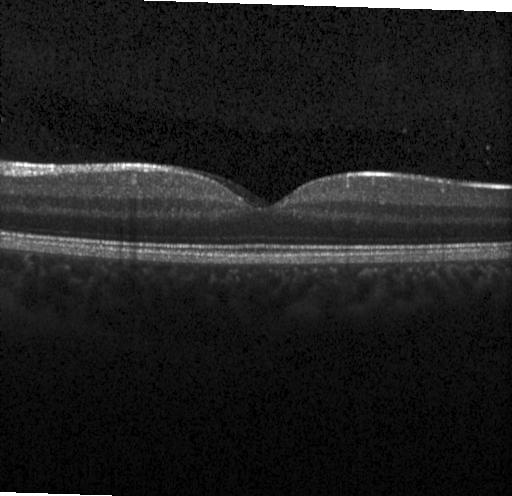 Spectral-domain optical coherence tomography · Heidelberg Spectralis OCT system · fovea-centered · optical coherence tomography B-scan
Impression: no choroidal neovascularization, diabetic macular edema, or drusen.